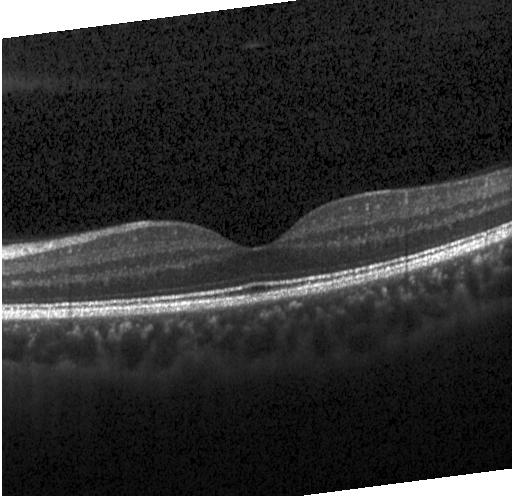
OCT B-scan showing neither choroidal neovascularization, diabetic macular edema, nor drusen.